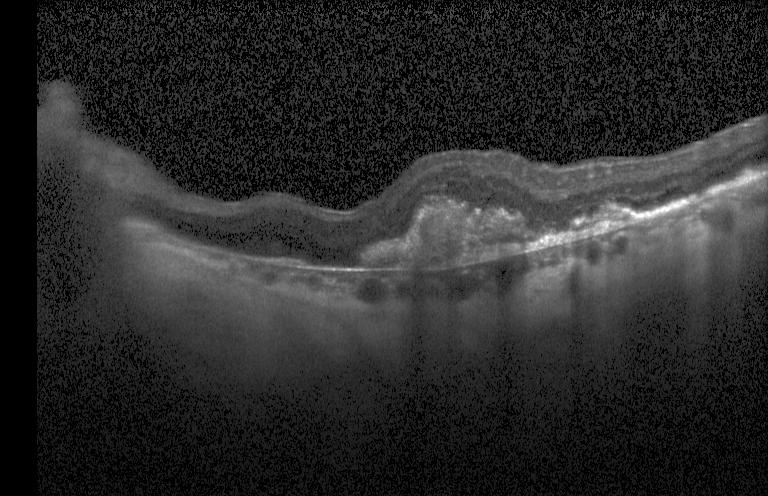
Heidelberg Spectralis OCT system · retinal OCT B-scan — Dx: a choroidal neovascular membrane.